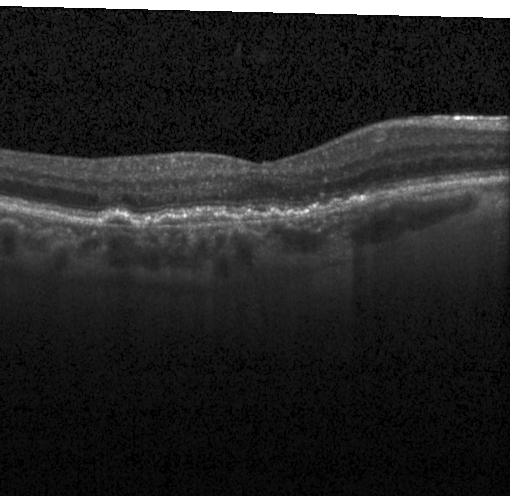
Instrument: Heidelberg Spectralis · spectral-domain optical coherence tomography · optical coherence tomography B-scan · macular scan. Assessment: CNV.